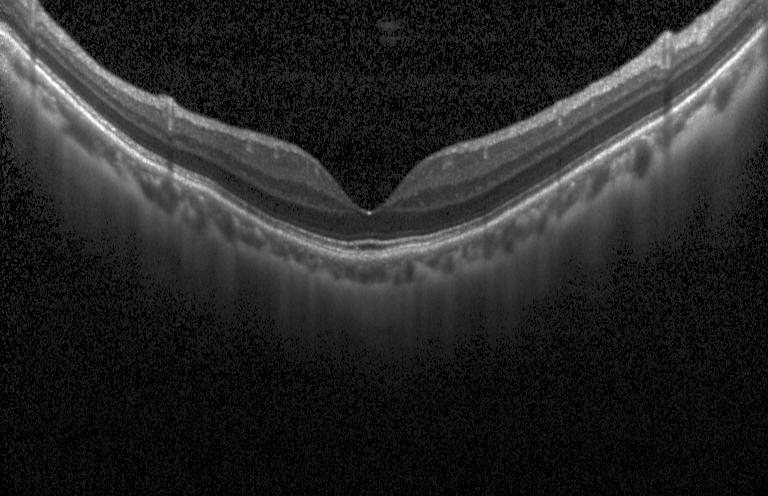

Retinal OCT cross-section; macular scan; spectral-domain optical coherence tomography; Heidelberg Spectralis OCT system. The scan shows no choroidal neovascularization, no diabetic macular edema, and no drusen.